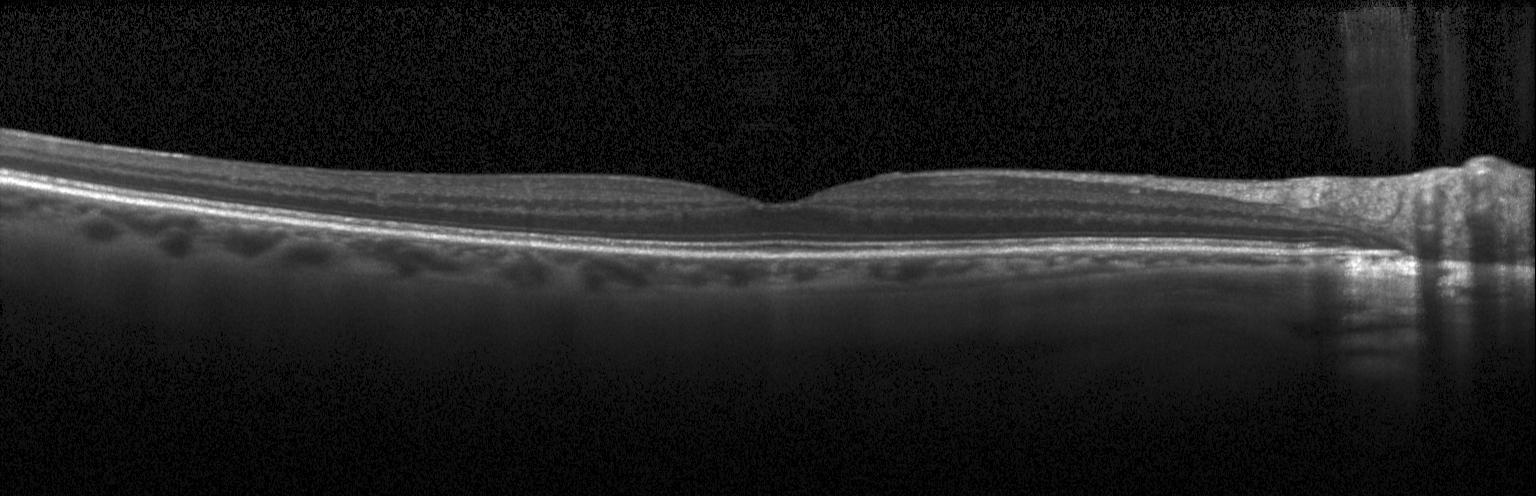 Optical coherence tomography B-scan. SD-OCT. OCT finding: no evidence of CNV, DME, or drusen.